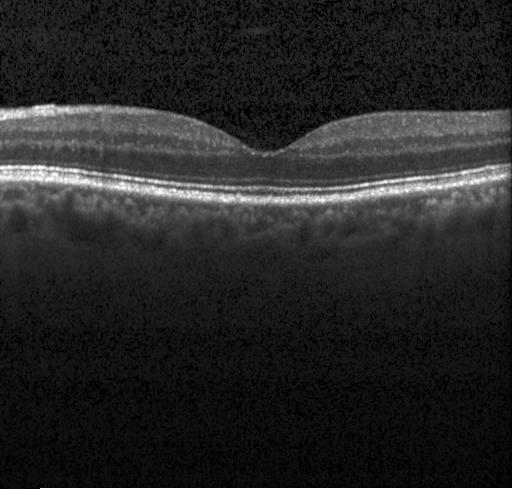

Spectral-domain OCT; retinal OCT B-scan — Finding: no choroidal neovascularization, no diabetic macular edema, and no drusen.